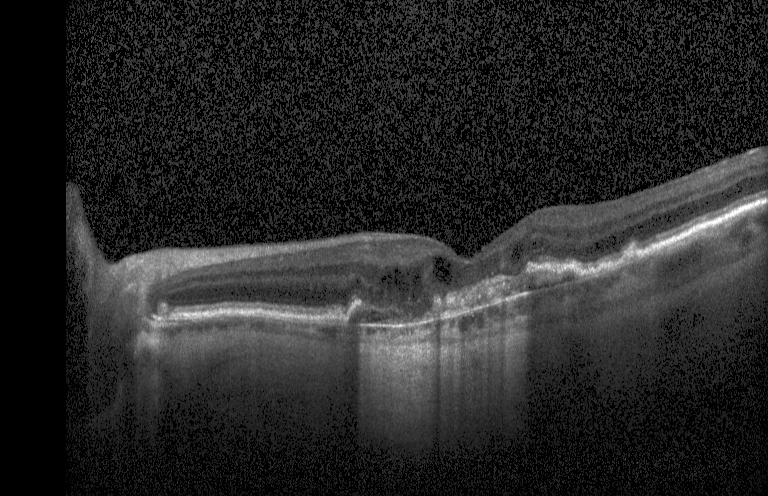

Retinal OCT cross-section · Heidelberg Spectralis. This B-scan demonstrates CNV.